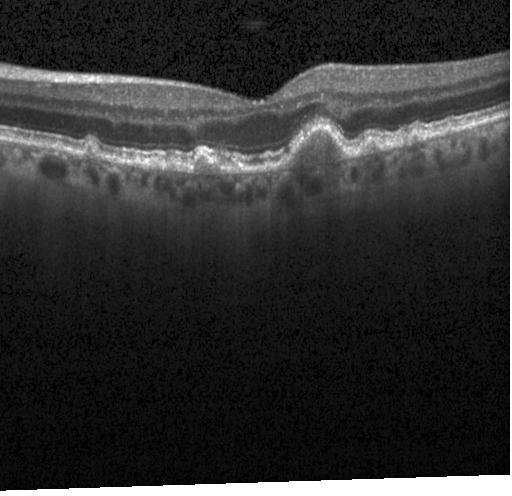
Retinal OCT B-scan · fovea-centered · instrument: Heidelberg Spectralis. Finding: sub-RPE drusenoid deposits.